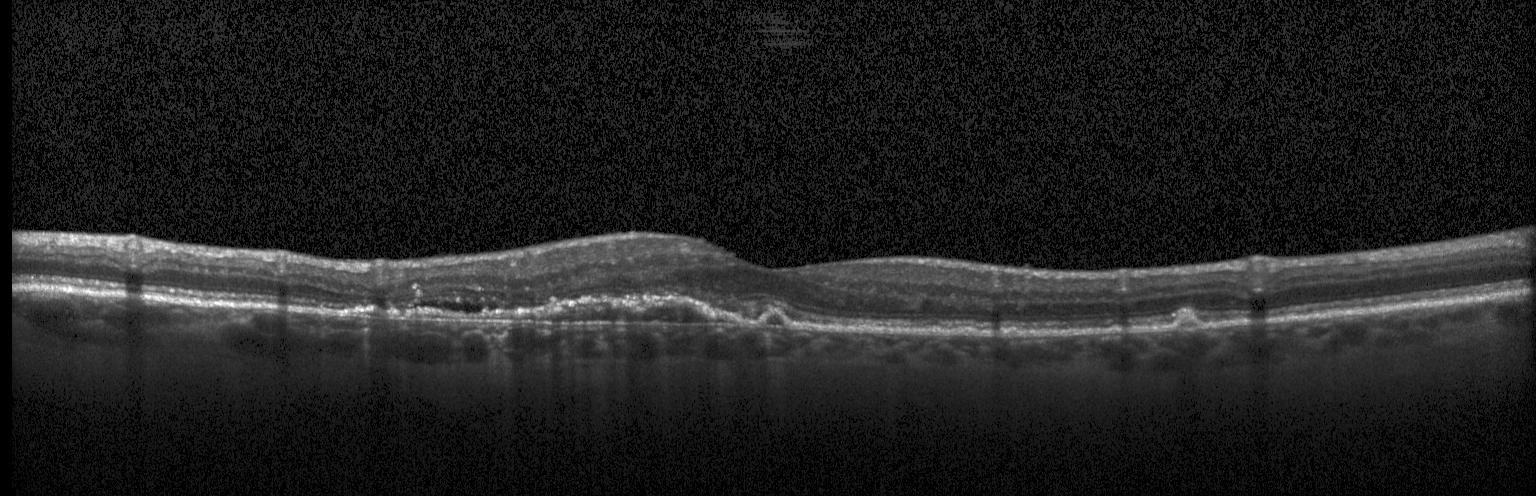
OCT finding: choroidal neovascularization.